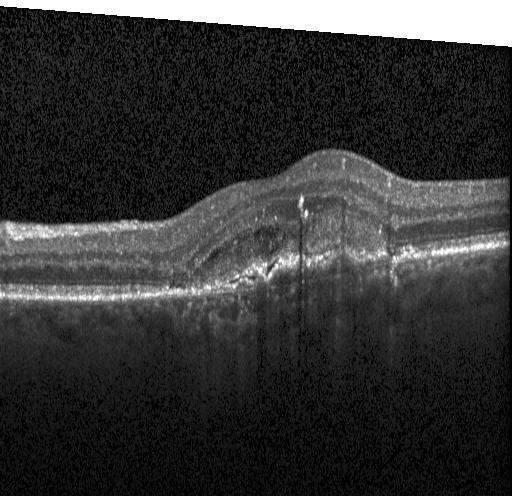
OCT finding: choroidal neovascularization.